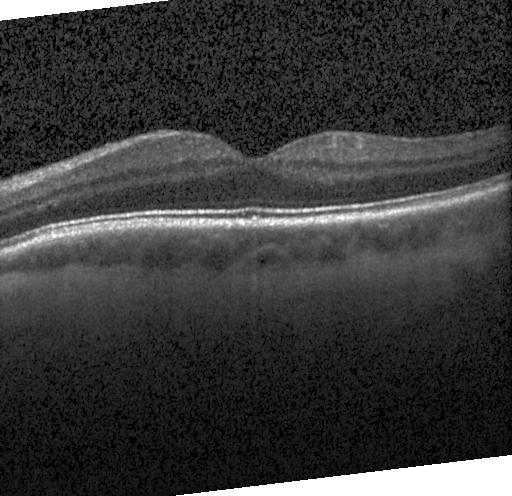

Fovea-centered. Spectral-domain optical coherence tomography. OCT line scan. OCT finding: no evidence of CNV, DME, or drusen.